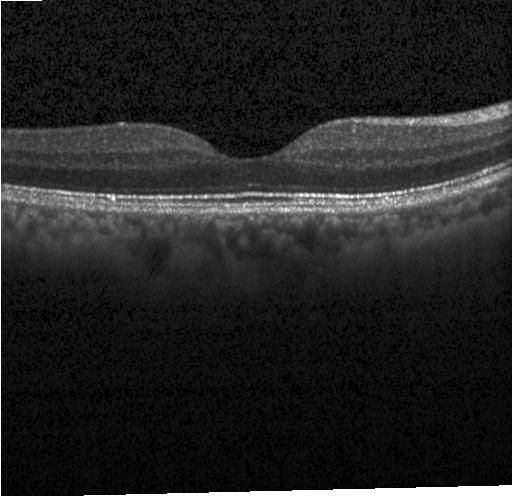

Centered on the fovea · optical coherence tomography B-scan · Heidelberg Spectralis OCT system · spectral-domain optical coherence tomography.
Dx: no evidence of CNV, DME, or drusen.